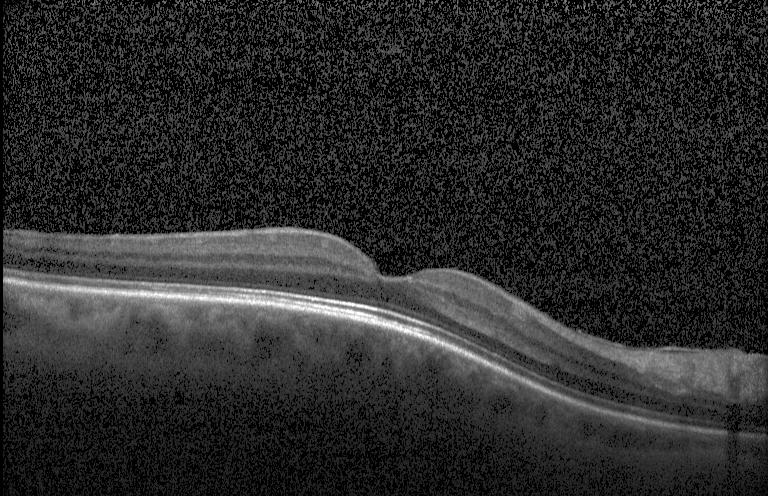
No choroidal neovascularization, no diabetic macular edema, and no drusen.